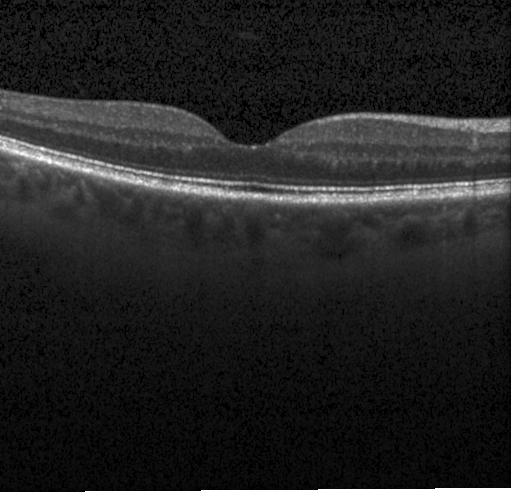
Heidelberg Spectralis OCT system; SD-OCT; optical coherence tomography scan; through the macula
Assessment: neither choroidal neovascularization, diabetic macular edema, nor drusen.